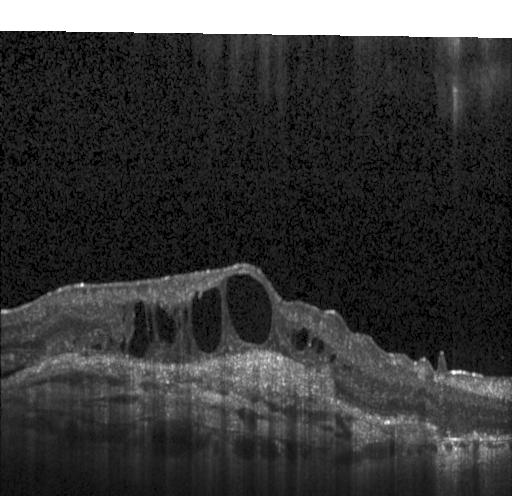

Retinal OCT cross-section showing CNV.